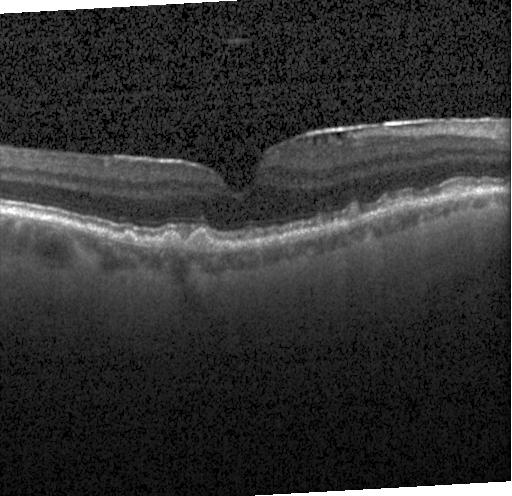
OCT B-scan.
This B-scan demonstrates drusen.